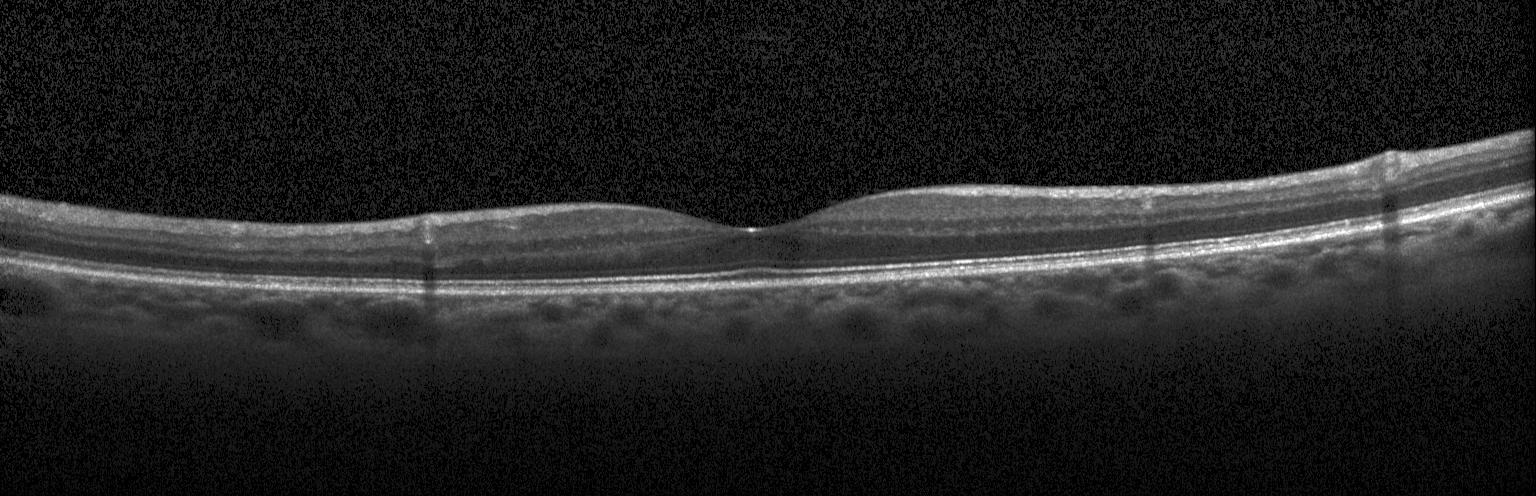
Fovea-centered; acquired on a Heidelberg Spectralis; spectral-domain optical coherence tomography; OCT line scan
OCT finding: no choroidal neovascularization, diabetic macular edema, or drusen.